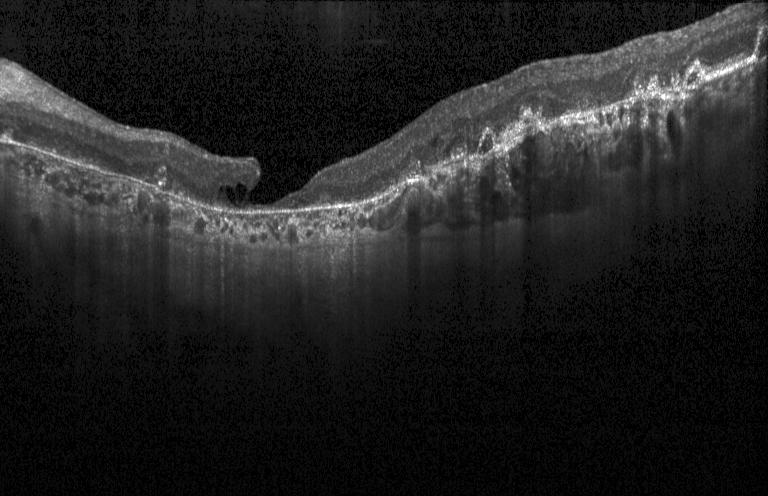
Instrument: Heidelberg Spectralis; optical coherence tomography scan — Finding: a choroidal neovascular membrane.